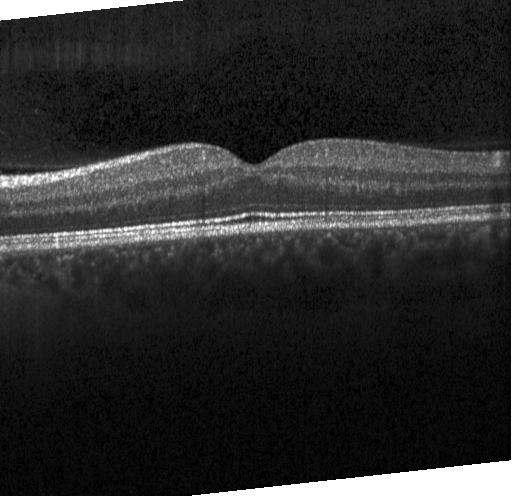

OCT scan showing no CNV, no DME, and no drusen.